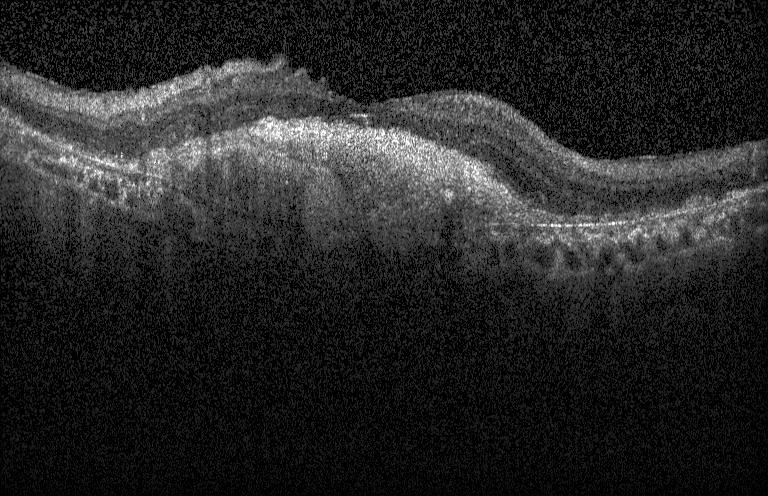
SD-OCT; optical coherence tomography B-scan; Heidelberg Spectralis OCT system — Dx: CNV.